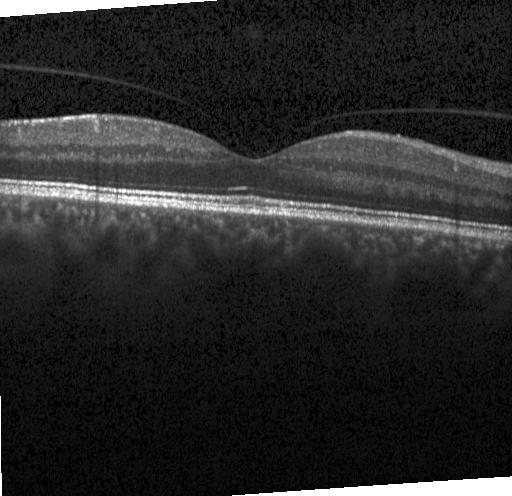 Diagnosis: no evidence of choroidal neovascularization, diabetic macular edema, or drusen.